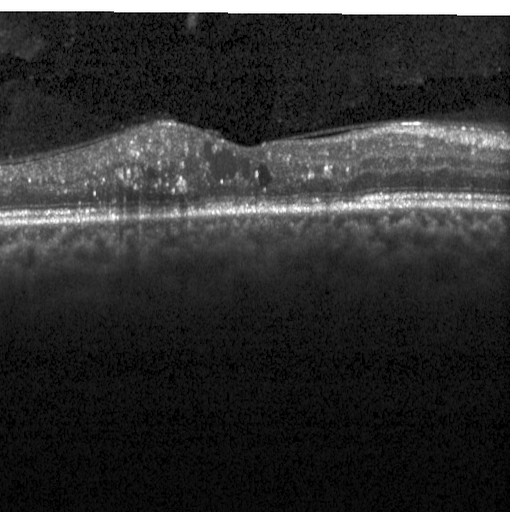

Heidelberg Spectralis; horizontal scan through the fovea; optical coherence tomography B-scan.
Assessment: diabetic macular edema.